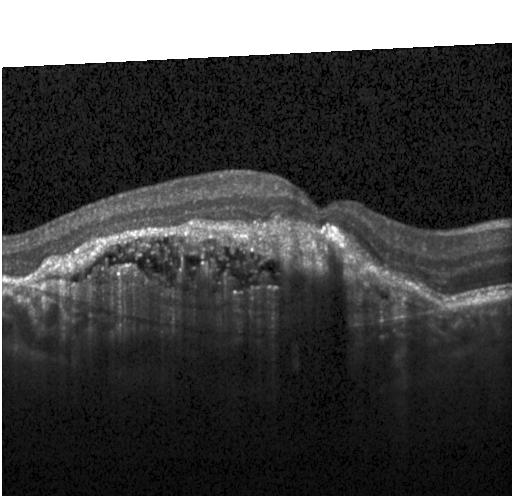
Impression: a choroidal neovascular membrane.